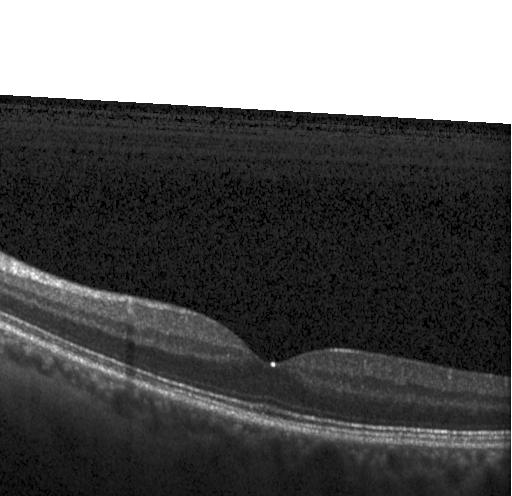

Retinal OCT B-scan; spectral-domain optical coherence tomography; instrument: Heidelberg Spectralis — This B-scan demonstrates no choroidal neovascularization, no diabetic macular edema, and no drusen.